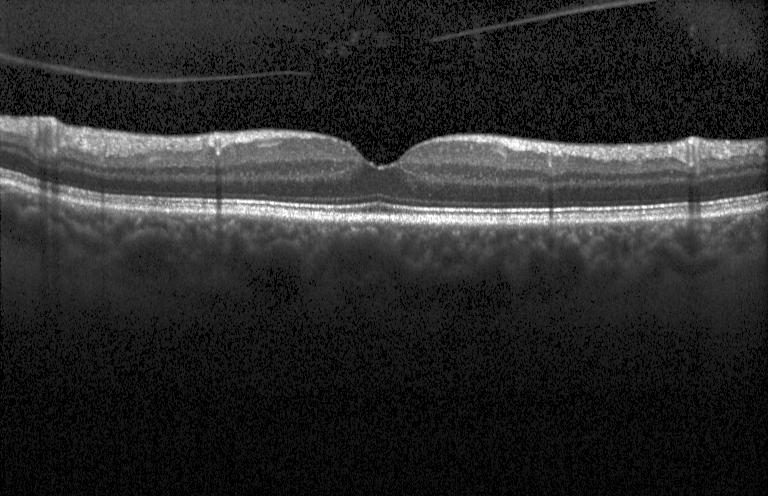 Macular OCT: no CNV, no DME, and no drusen.